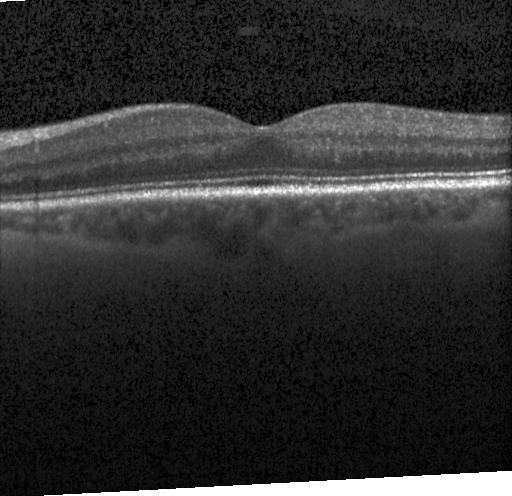

Impression: no choroidal neovascularization, no diabetic macular edema, and no drusen.